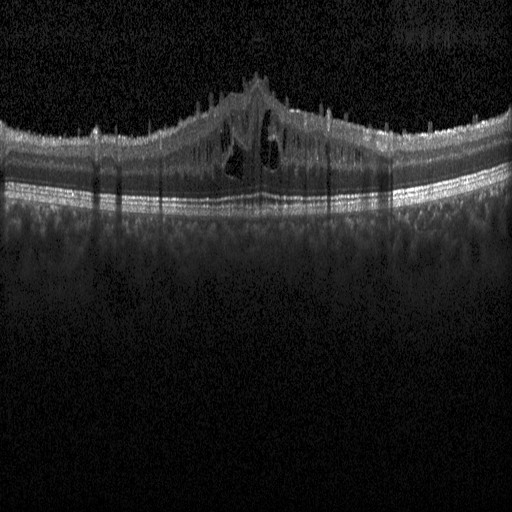 OCT B-scan, macular scan, spectral-domain optical coherence tomography — Assessment: DME.